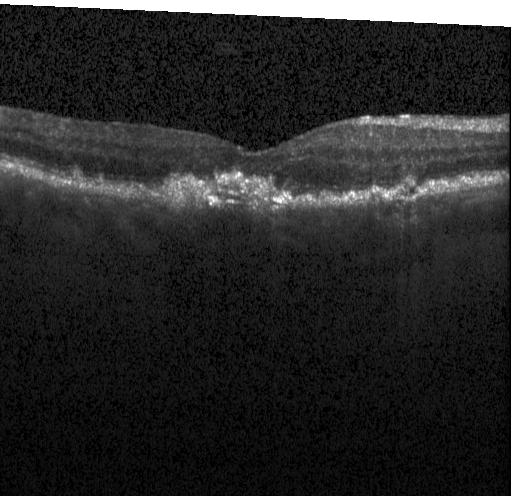
Retinal OCT B-scan — Macular OCT: CNV.